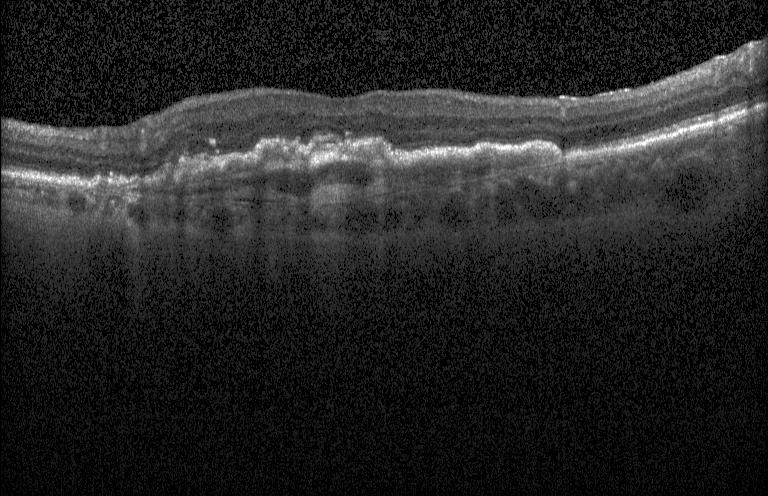
Heidelberg Spectralis OCT system. OCT line scan
A choroidal neovascular membrane.